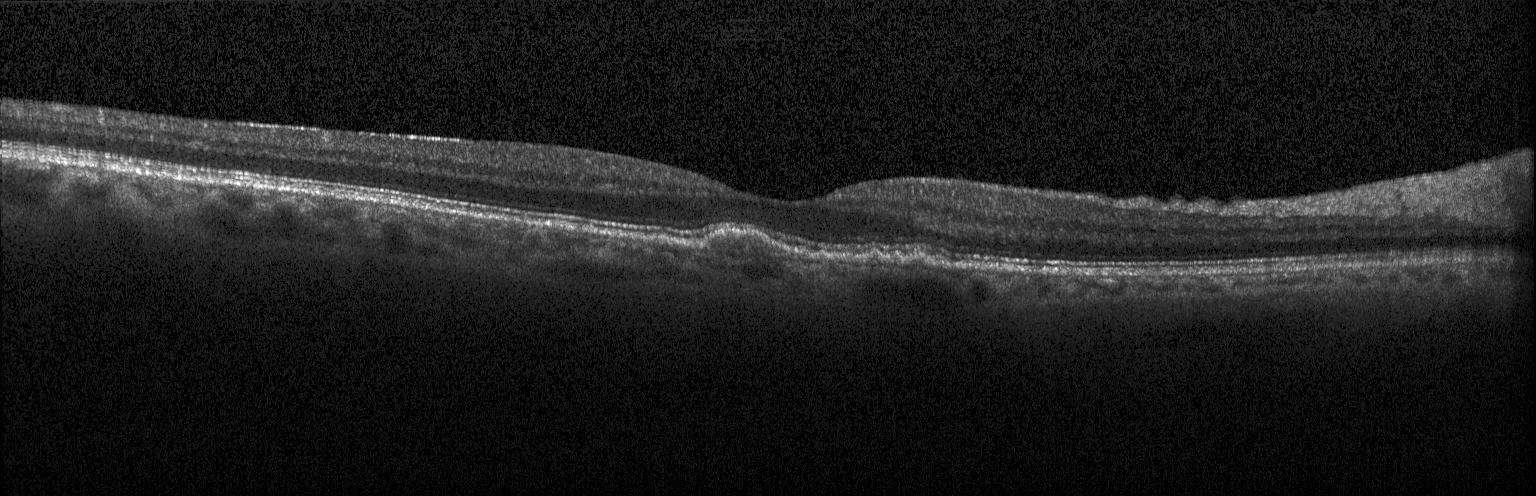
Assessment: drusen.